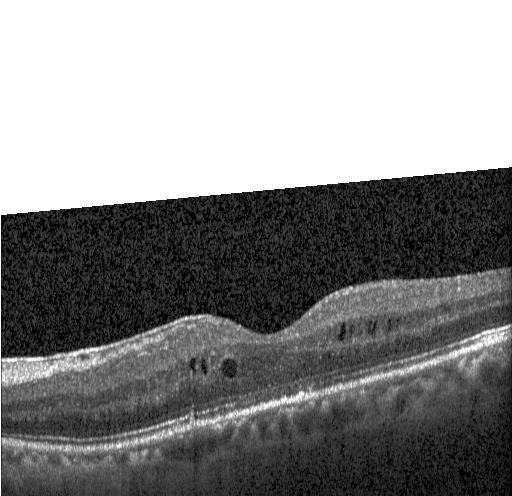

Optical coherence tomography B-scan.
Assessment: diabetic macular edema (DME).